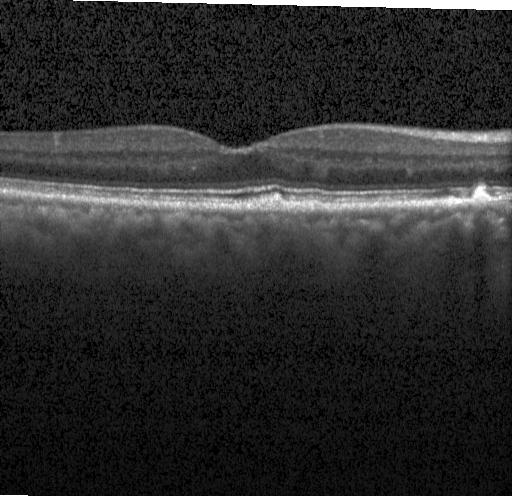 Centered on the fovea · SD-OCT · OCT B-scan — The scan shows sub-RPE drusenoid deposits.